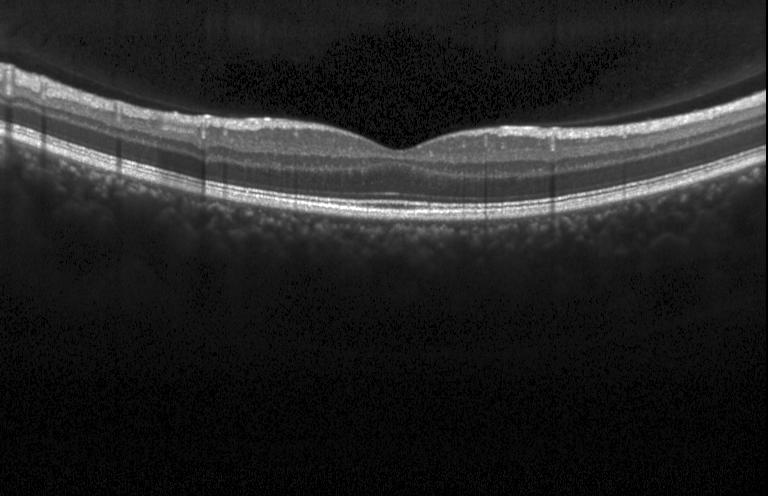

Retinal OCT cross-section — Impression: no choroidal neovascularization, diabetic macular edema, or drusen.